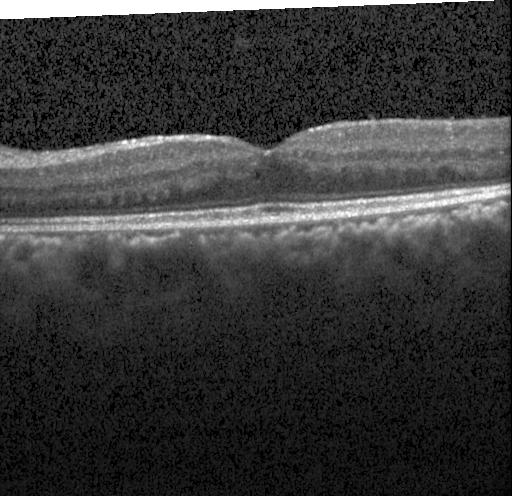 Retinal OCT B-scan; SD-OCT
Finding: diabetic macular edema (DME).